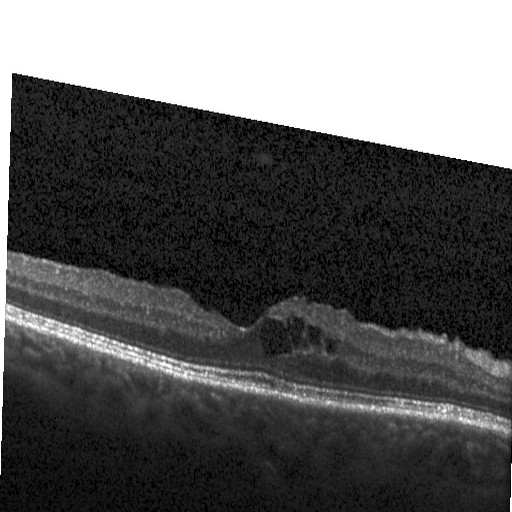
Diabetic macular edema (DME).